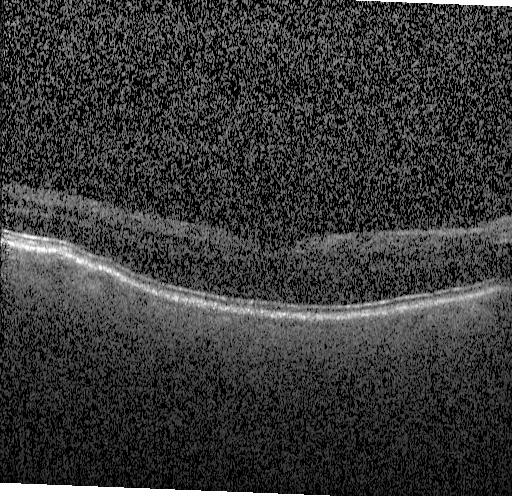

OCT scan showing no CNV, DME, or drusen.